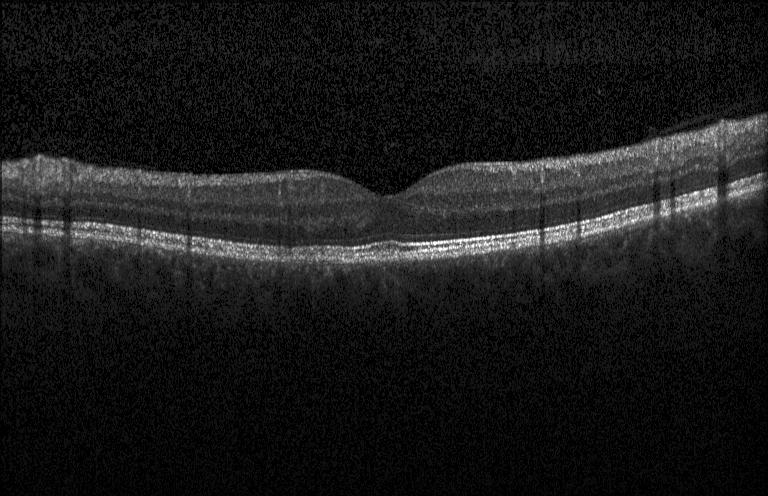
Spectral-domain OCT · acquired on a Heidelberg Spectralis · optical coherence tomography B-scan · centered on the fovea — Neither choroidal neovascularization, diabetic macular edema, nor drusen.